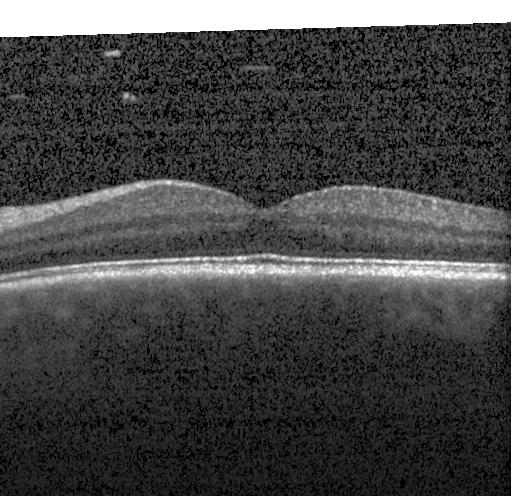 Fovea-centered · SD-OCT · Heidelberg Spectralis · optical coherence tomography B-scan
Finding: no CNV, no DME, and no drusen.